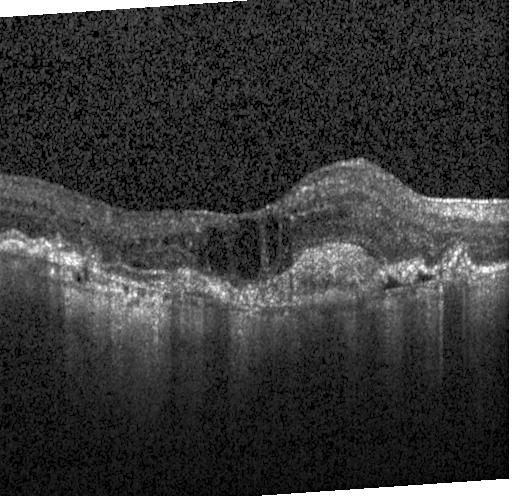 Spectral-domain optical coherence tomography, optical coherence tomography scan, macular scan, instrument: Heidelberg Spectralis. A choroidal neovascular membrane.